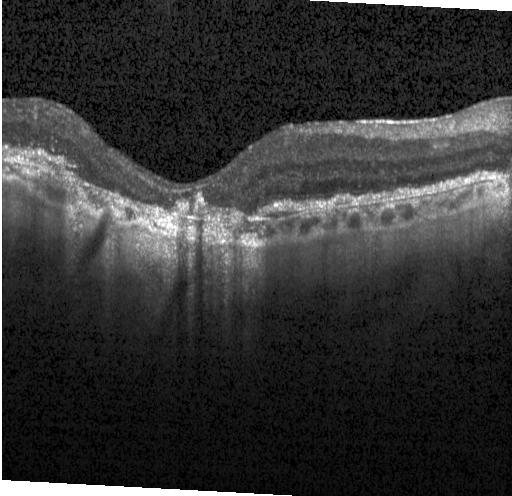 Impression: CNV.